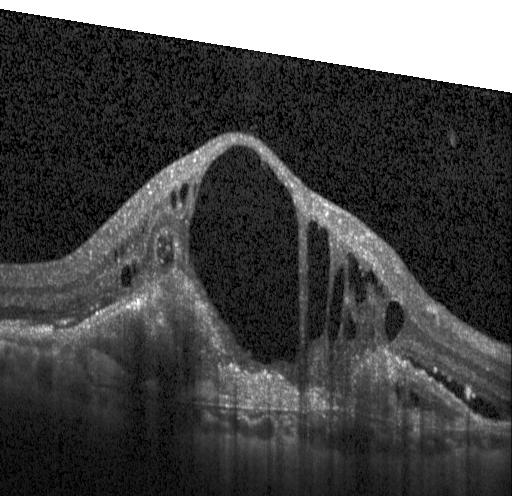
Macular scan; instrument: Heidelberg Spectralis; retinal OCT B-scan; spectral-domain optical coherence tomography.
Finding: choroidal neovascularization (CNV).